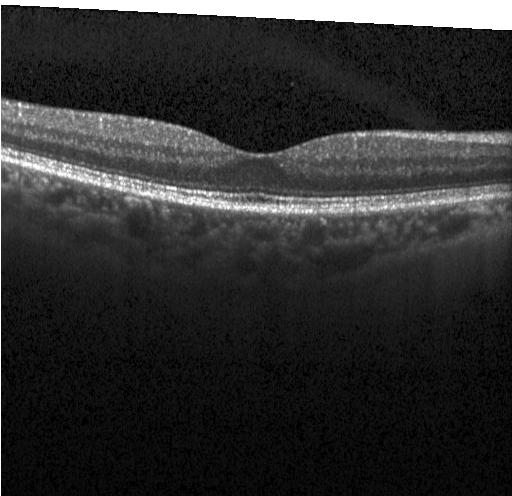
OCT B-scan showing no choroidal neovascularization, no diabetic macular edema, and no drusen.